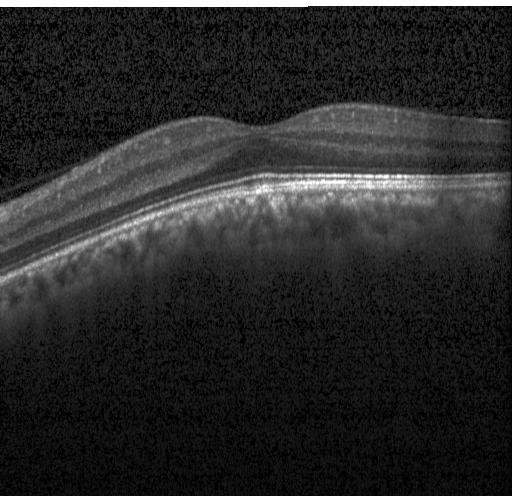 Centered on the fovea. Optical coherence tomography B-scan. Acquired on a Heidelberg Spectralis. No choroidal neovascularization, no diabetic macular edema, and no drusen.